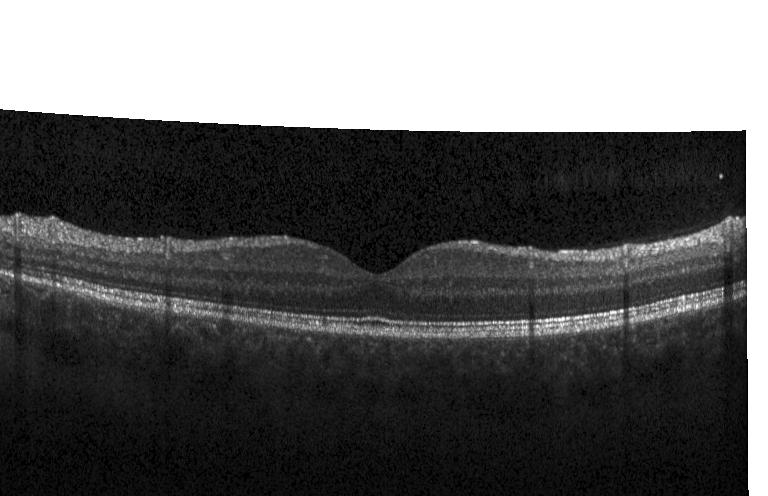
Through the macula · OCT B-scan · acquired on a Heidelberg Spectralis
Finding: no choroidal neovascularization, no diabetic macular edema, and no drusen.